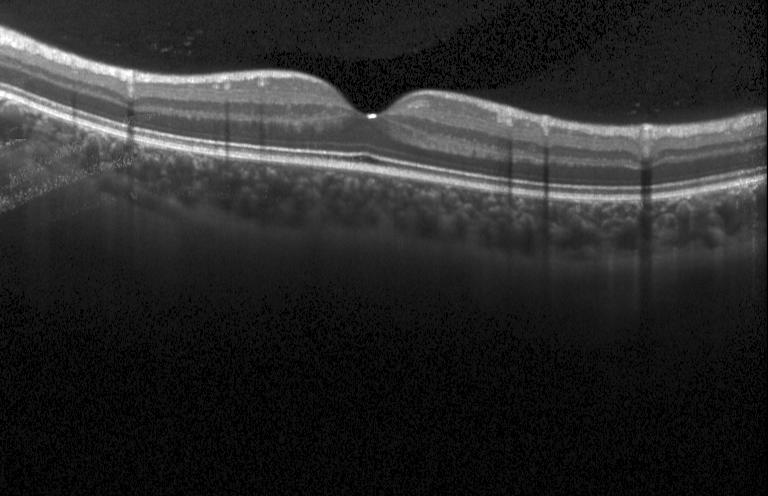
Retinal OCT B-scan; centered on the fovea; SD-OCT
Finding: no CNV, DME, or drusen.